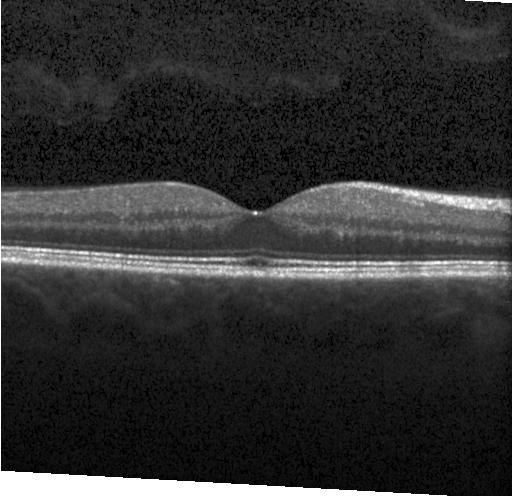

Impression: no choroidal neovascularization, no diabetic macular edema, and no drusen.